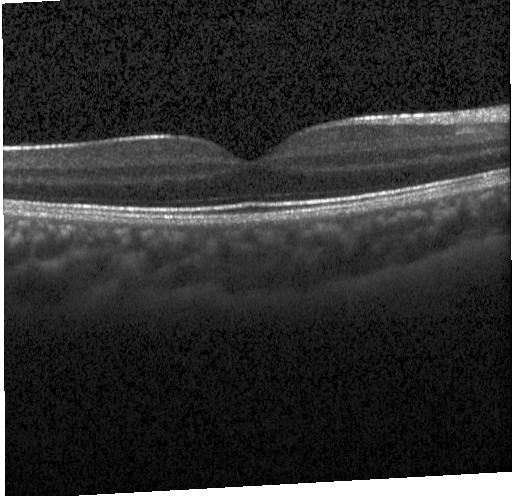 Spectral-domain OCT B-scan: no choroidal neovascularization, diabetic macular edema, or drusen.